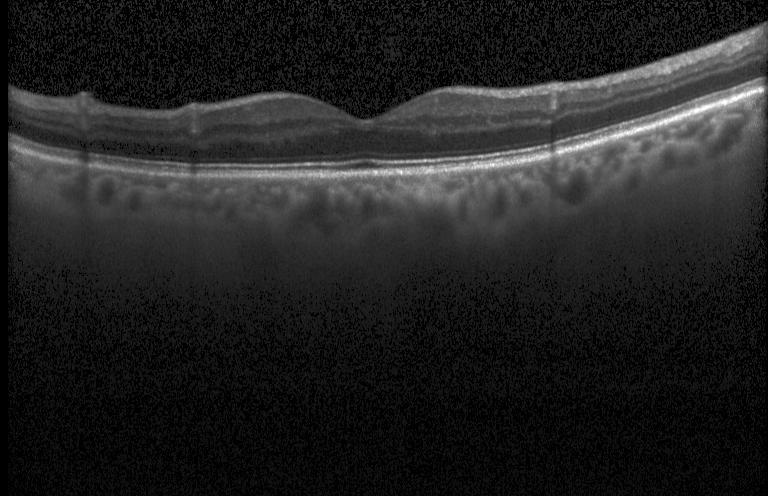
Acquired on a Heidelberg Spectralis; optical coherence tomography B-scan; spectral-domain optical coherence tomography — OCT finding: no CNV, no DME, and no drusen.